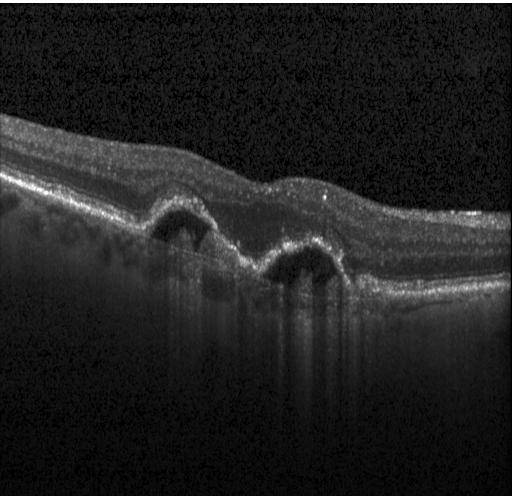 OCT B-scan
OCT finding: a choroidal neovascular membrane.